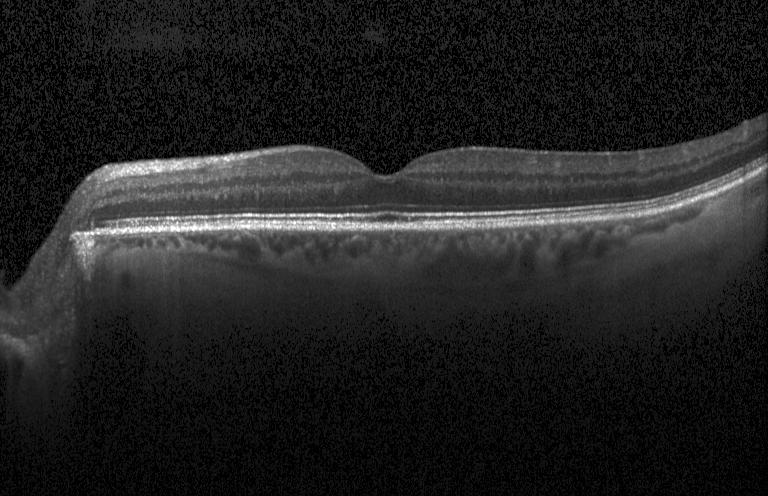
Dx: no evidence of choroidal neovascularization, diabetic macular edema, or drusen.